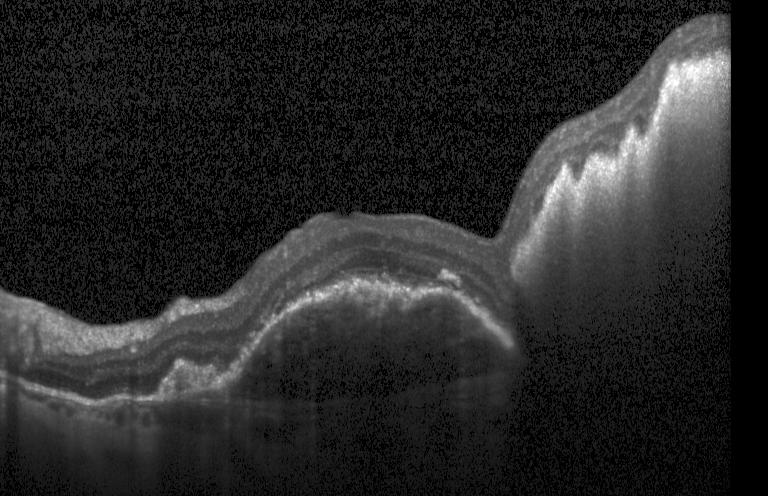 Retinal OCT cross-section showing a choroidal neovascular membrane.